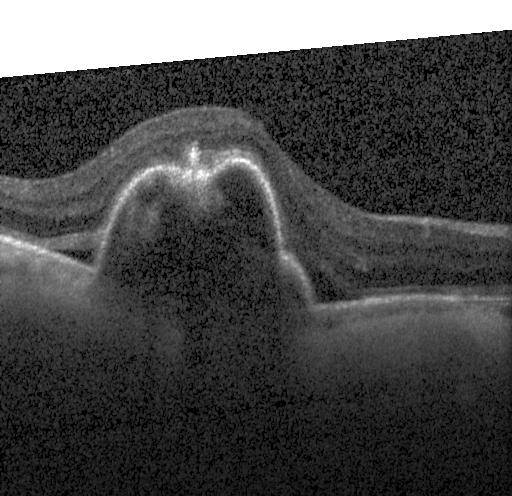 OCT B-scan · horizontal scan through the fovea · spectral-domain optical coherence tomography.
OCT finding: choroidal neovascularization (CNV).